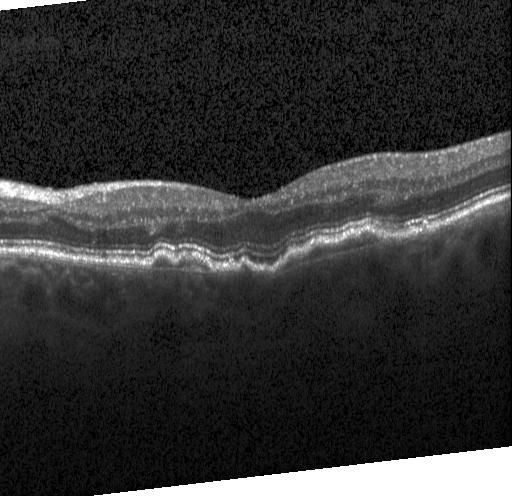 Retinal OCT B-scan, spectral-domain optical coherence tomography
This B-scan demonstrates CNV.